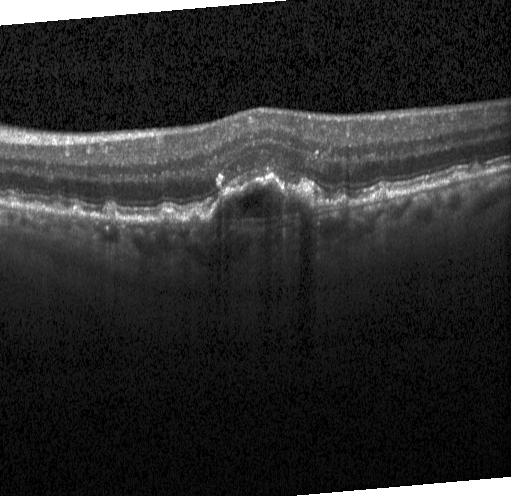

Dx: a choroidal neovascular membrane.